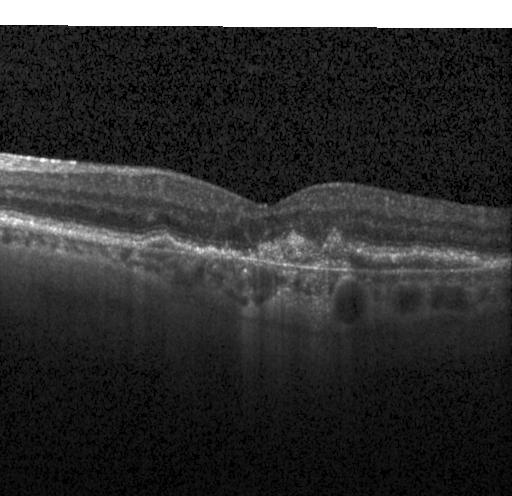 Heidelberg Spectralis OCT system, OCT line scan, fovea-centered.
Impression: choroidal neovascularization.